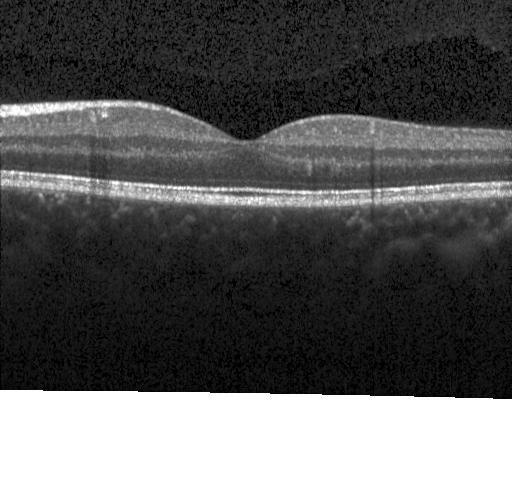 Optical coherence tomography B-scan, spectral-domain optical coherence tomography, Heidelberg Spectralis
Finding: no choroidal neovascularization, no diabetic macular edema, and no drusen.